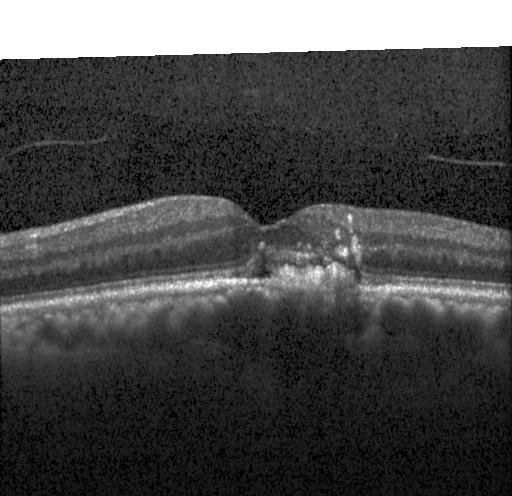 Optical coherence tomography B-scan — A choroidal neovascular membrane.